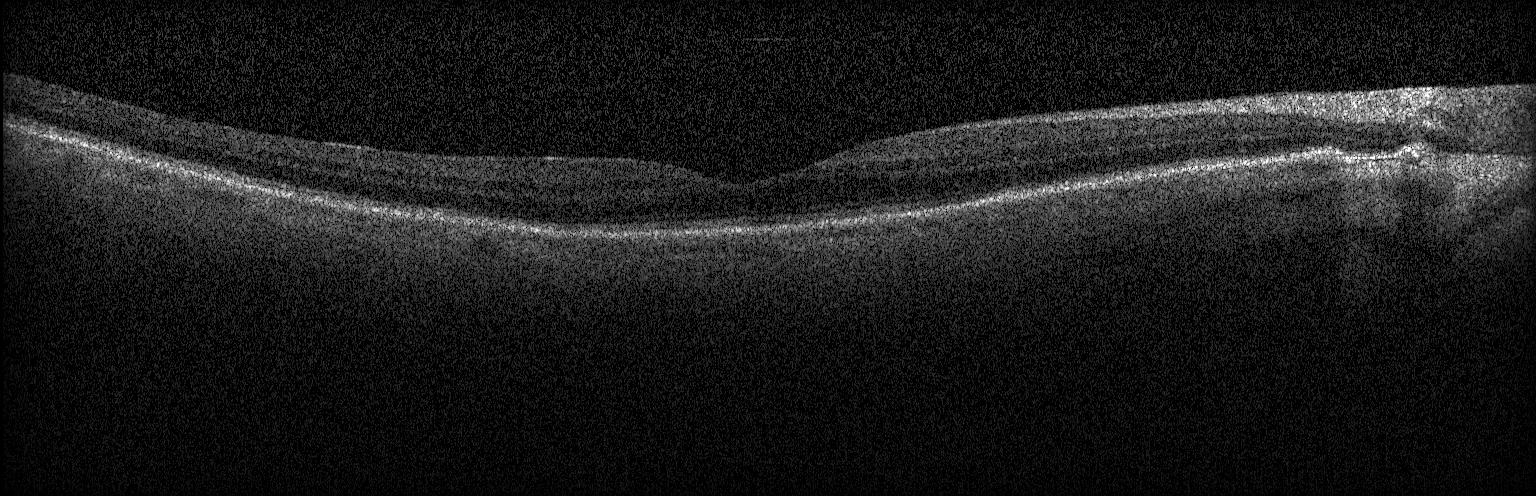

Retinal OCT B-scan · spectral-domain optical coherence tomography · macular scan · Heidelberg Spectralis OCT system.
Macular OCT: no evidence of CNV, DME, or drusen.